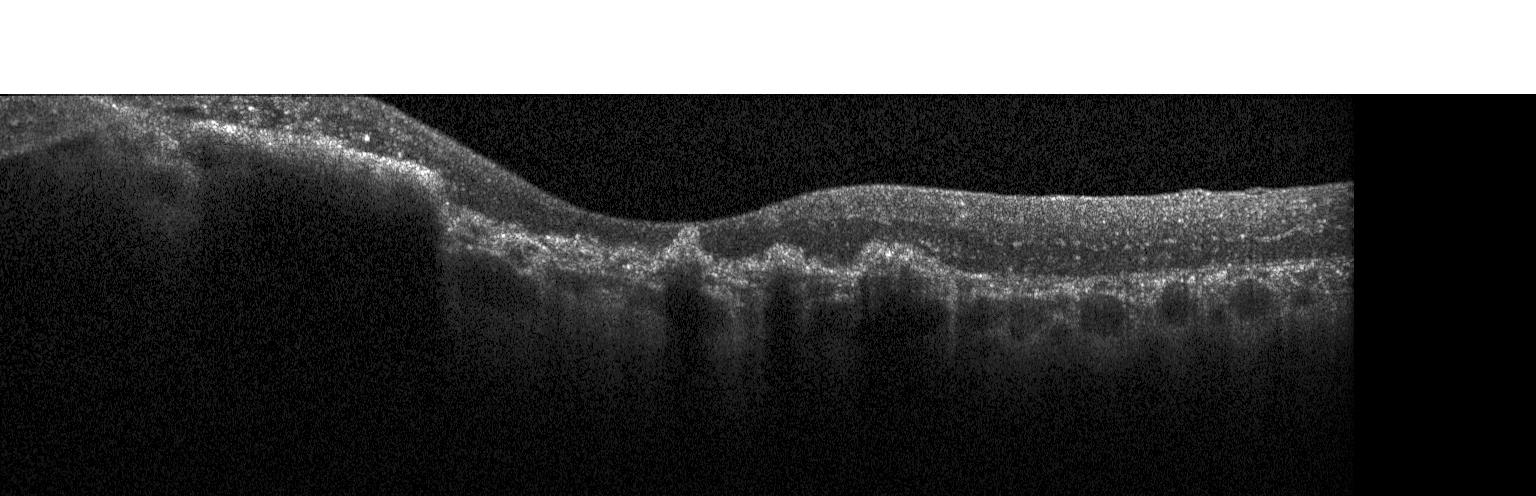
Spectral-domain optical coherence tomography · OCT B-scan · centered on the fovea · Heidelberg Spectralis
Impression: a choroidal neovascular membrane.